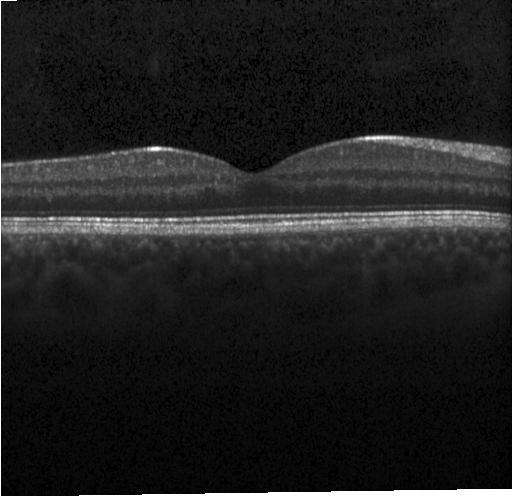 Finding: no evidence of choroidal neovascularization, diabetic macular edema, or drusen.